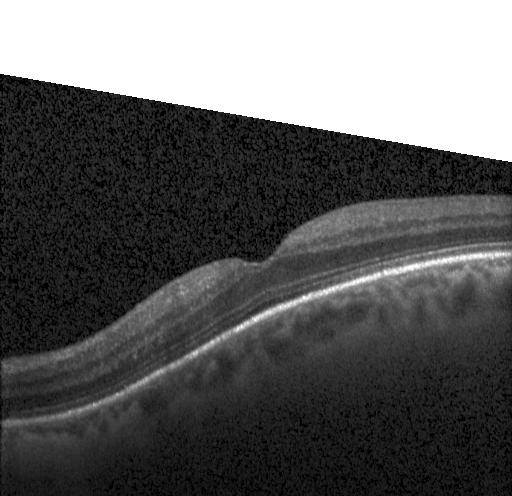 Finding: neither choroidal neovascularization, diabetic macular edema, nor drusen.